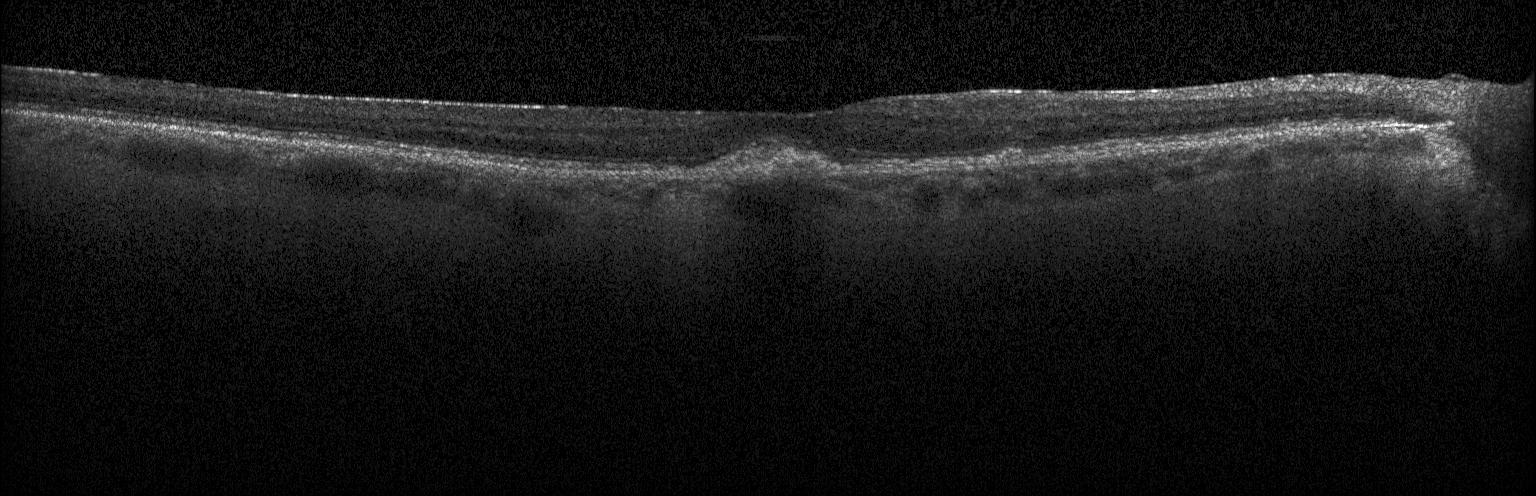

Heidelberg Spectralis OCT system. Optical coherence tomography B-scan. Horizontal scan through the fovea
The scan shows CNV.